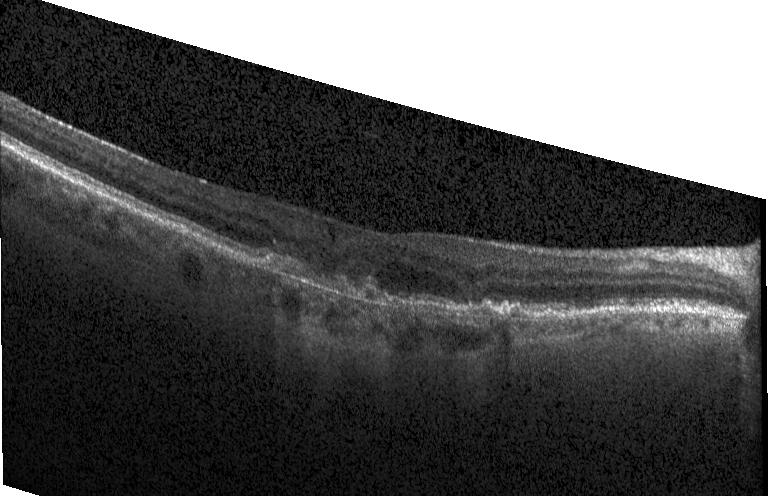

Finding: a choroidal neovascular membrane.